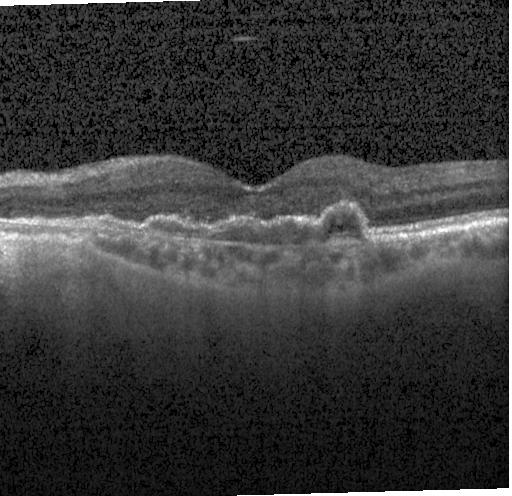

Spectral-domain optical coherence tomography · retinal OCT cross-section · centered on the fovea
Impression: choroidal neovascularization.